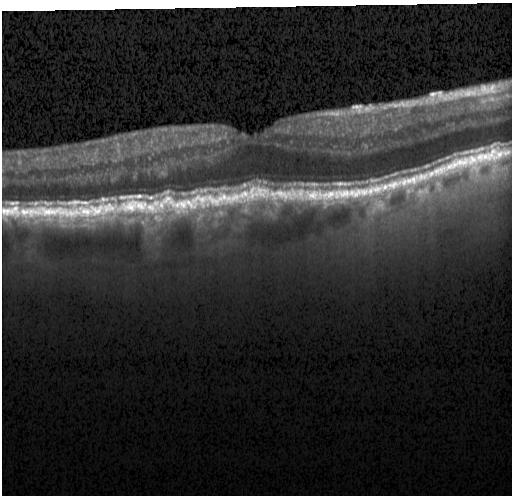 Optical coherence tomography scan; spectral-domain optical coherence tomography; instrument: Heidelberg Spectralis — Multiple drusen.